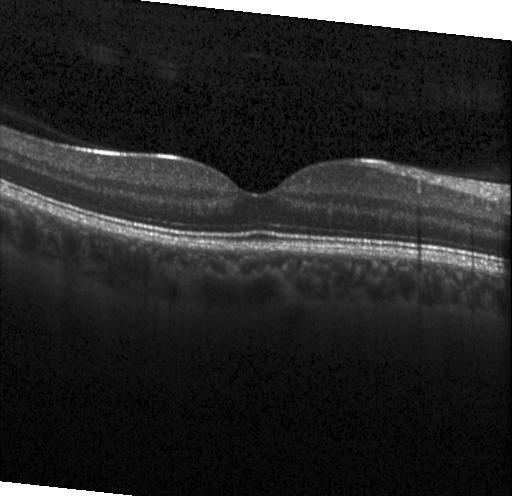 No CNV, DME, or drusen.